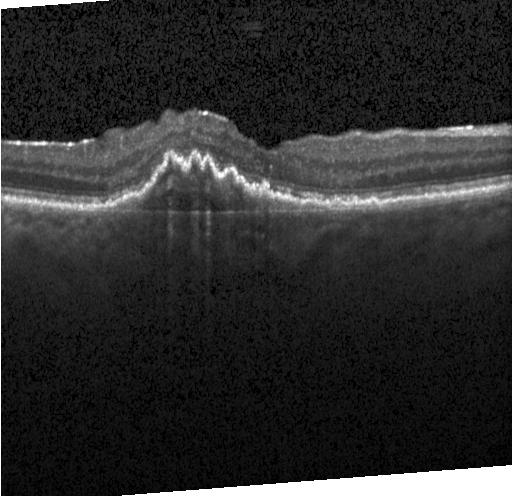
Optical coherence tomography scan. Fovea-centered. Finding: a choroidal neovascular membrane.